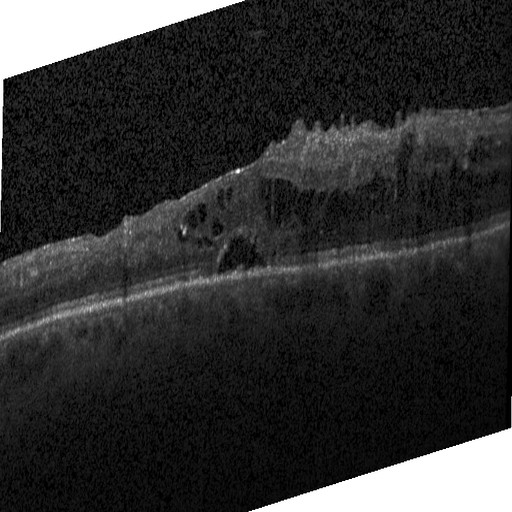

Dx: DME.